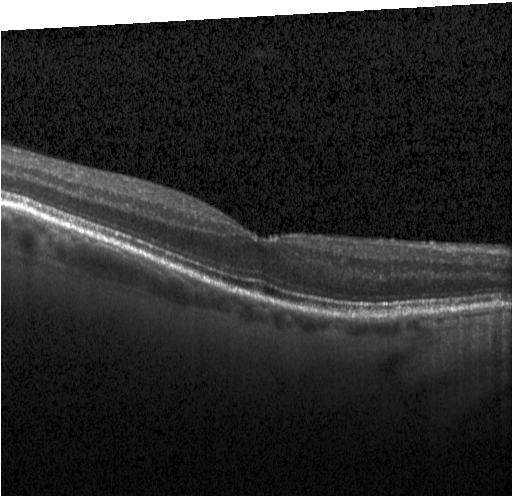

Spectral-domain optical coherence tomography, Heidelberg Spectralis, centered on the fovea, retinal OCT B-scan. Finding: no CNV, DME, or drusen.